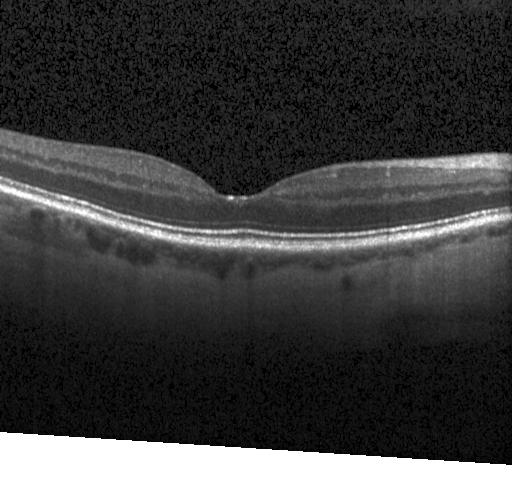
Heidelberg Spectralis OCT system; OCT B-scan — Finding: neither CNV, DME, nor drusen.